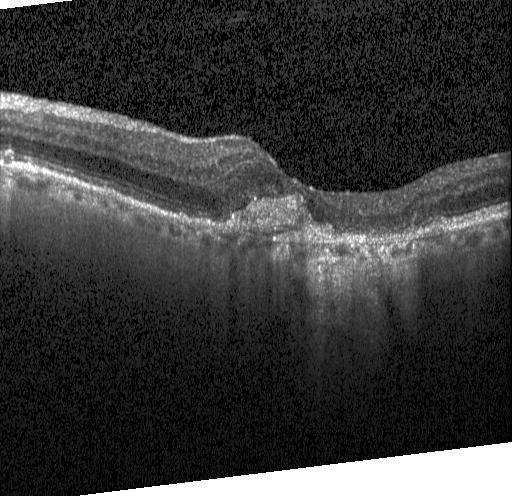
OCT line scan
Finding: a choroidal neovascular membrane.